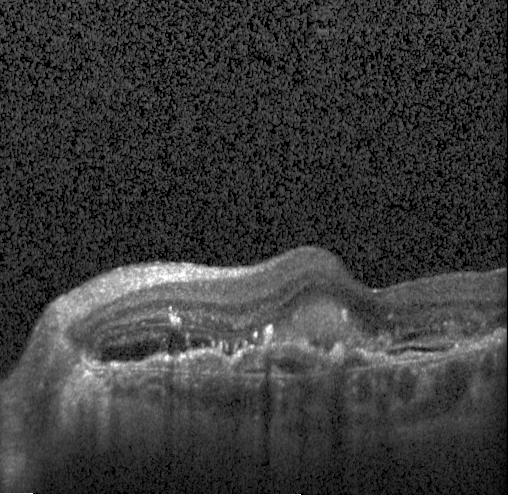 Centered on the fovea; OCT line scan; Heidelberg Spectralis OCT system
Assessment: choroidal neovascularization (CNV).